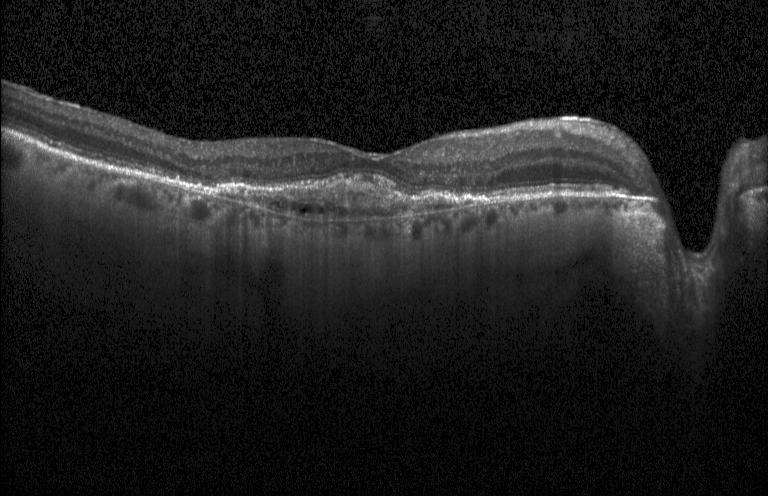
Macular OCT demonstrating a choroidal neovascular membrane.